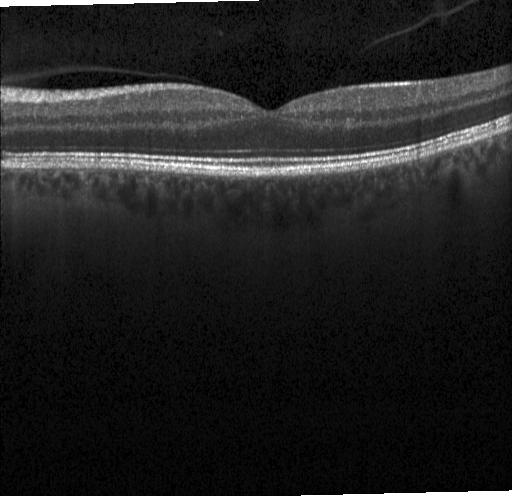
Centered on the fovea. OCT line scan
Neither choroidal neovascularization, diabetic macular edema, nor drusen.